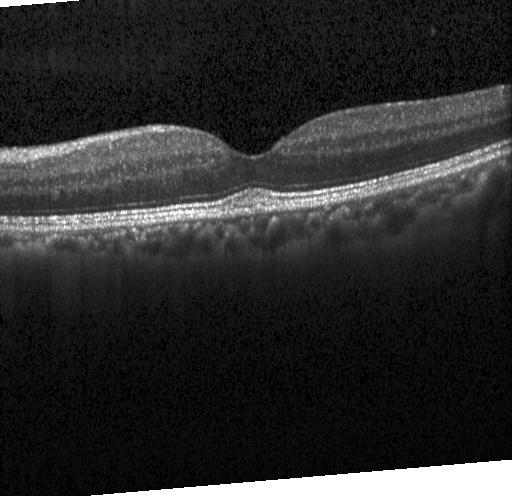

Finding: no choroidal neovascularization, diabetic macular edema, or drusen.